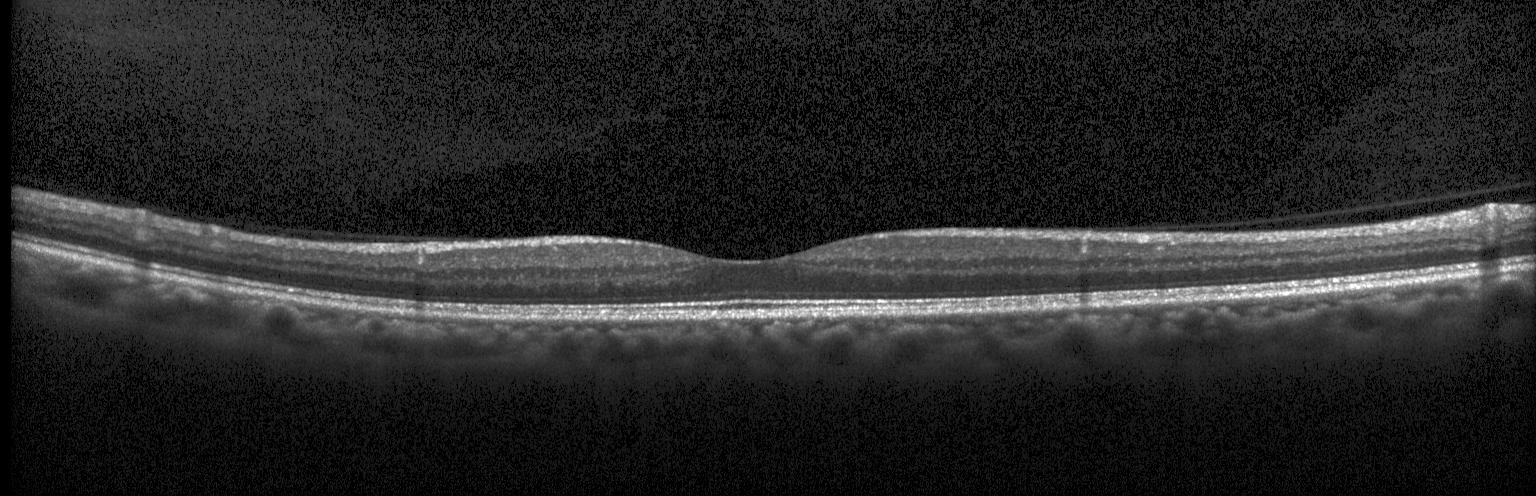

Retinal OCT cross-section · acquired on a Heidelberg Spectralis · SD-OCT · macular scan.
Assessment: no evidence of choroidal neovascularization, diabetic macular edema, or drusen.